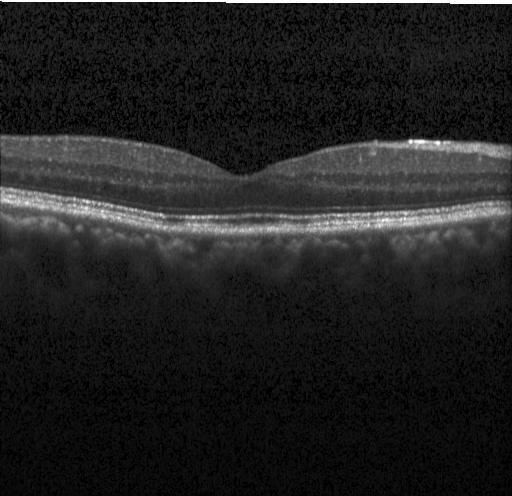
Macular scan, SD-OCT, OCT line scan. Impression: no choroidal neovascularization, no diabetic macular edema, and no drusen.